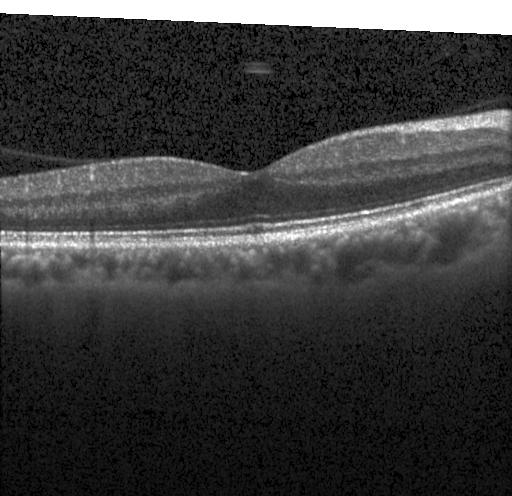
Horizontal scan through the fovea. Acquired on a Heidelberg Spectralis. Spectral-domain OCT. Optical coherence tomography B-scan. Finding: neither choroidal neovascularization, diabetic macular edema, nor drusen.